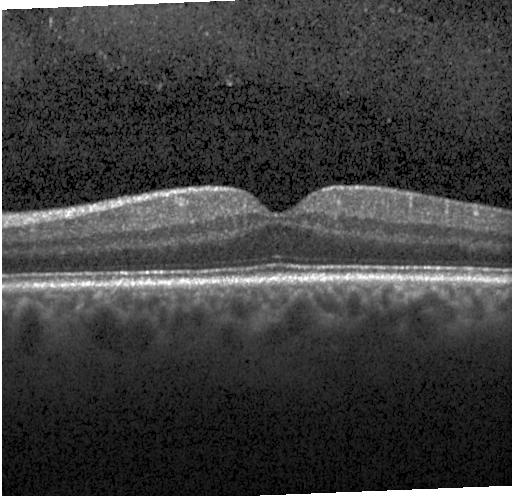 Heidelberg Spectralis OCT system · SD-OCT · horizontal scan through the fovea · retinal OCT B-scan.
Finding: no CNV, no DME, and no drusen.